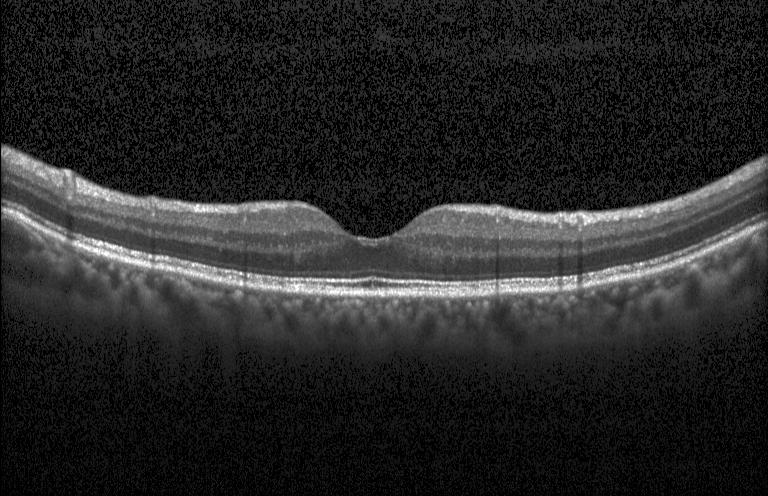 OCT B-scan. Dx: no choroidal neovascularization, diabetic macular edema, or drusen.